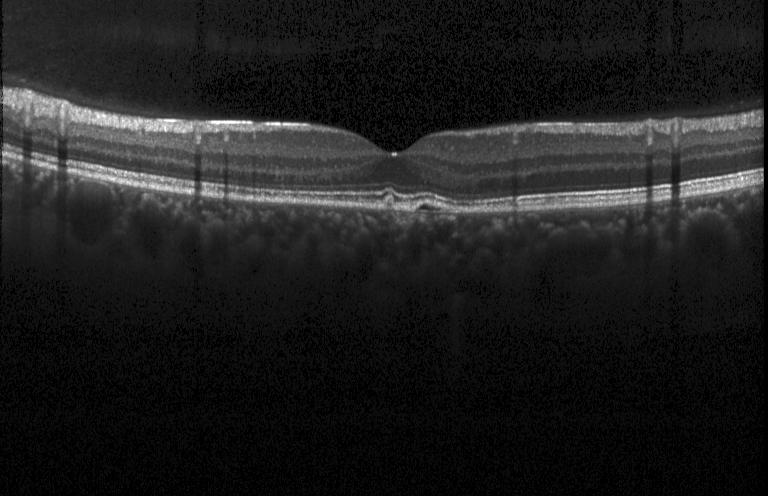 OCT line scan. Through the macula.
OCT finding: drusen.